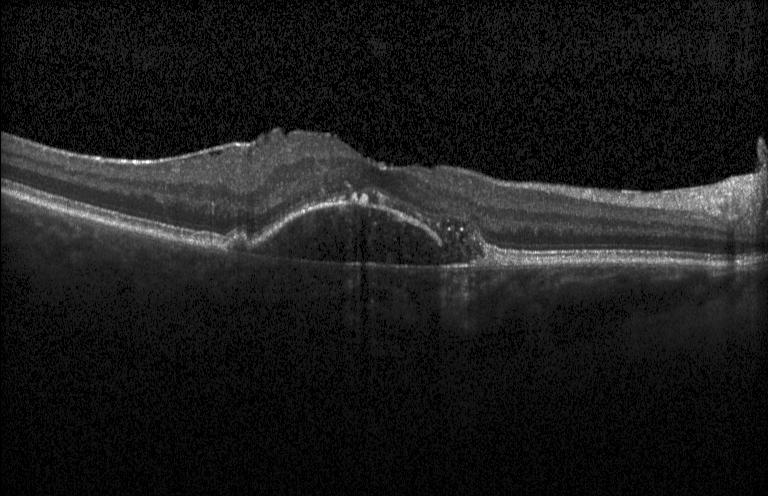 Retinal OCT cross-section. Acquired on a Heidelberg Spectralis — Diagnosis: CNV.